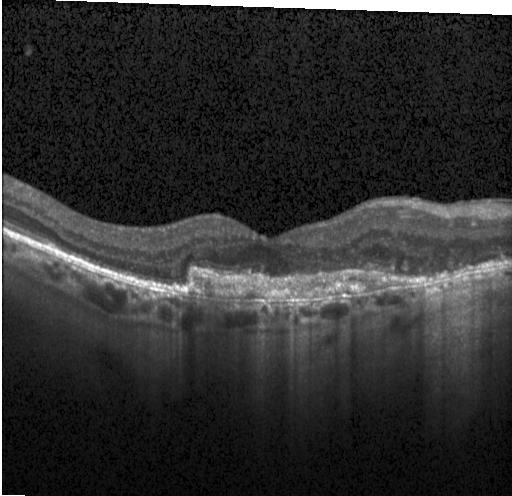 Dx: a choroidal neovascular membrane.